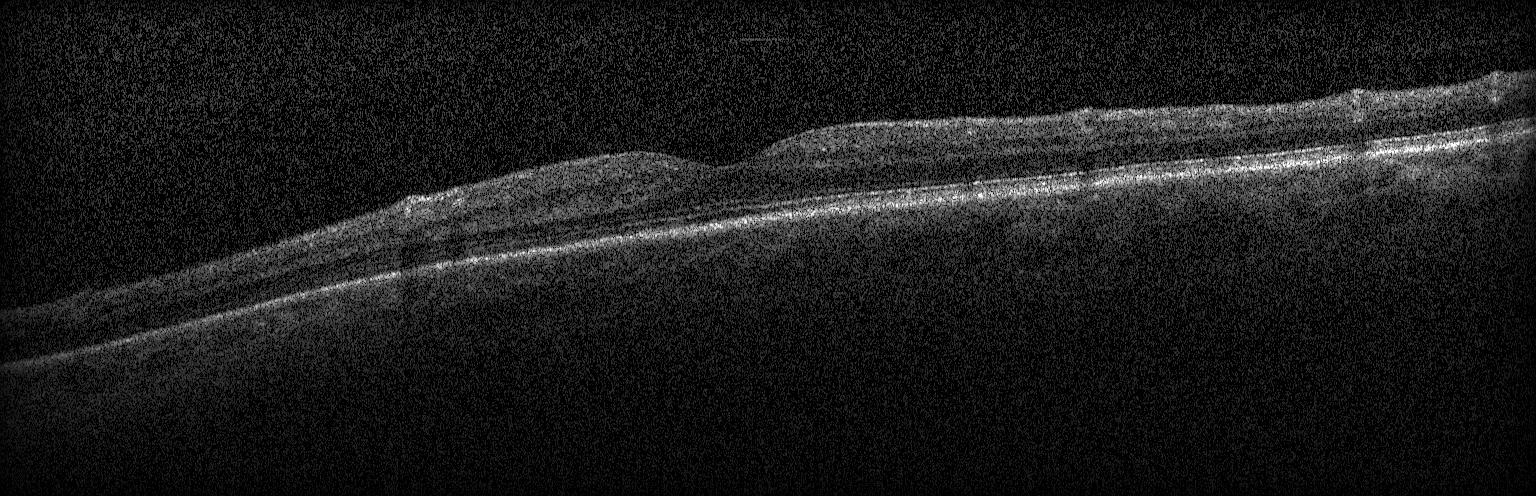 Macular OCT demonstrating no evidence of choroidal neovascularization, diabetic macular edema, or drusen.